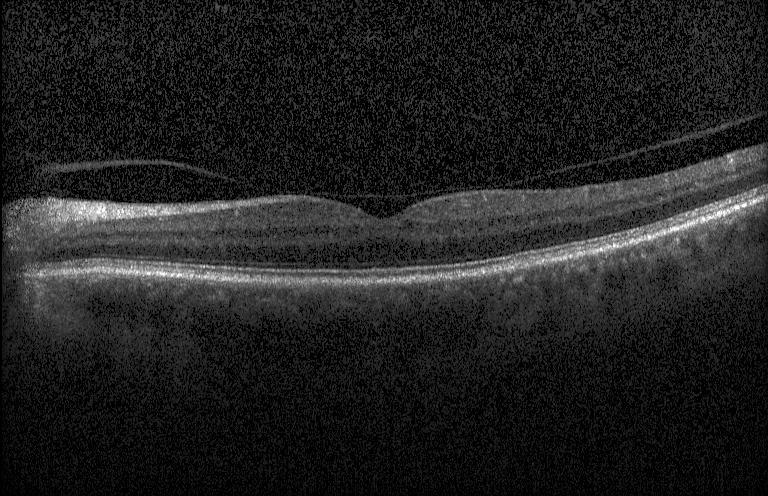 Retinal OCT cross-section.
OCT finding: neither choroidal neovascularization, diabetic macular edema, nor drusen.